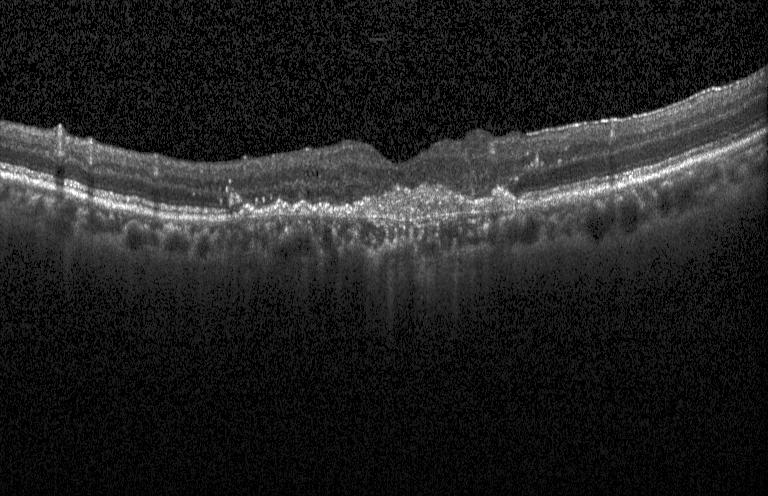
Dx: a choroidal neovascular membrane.